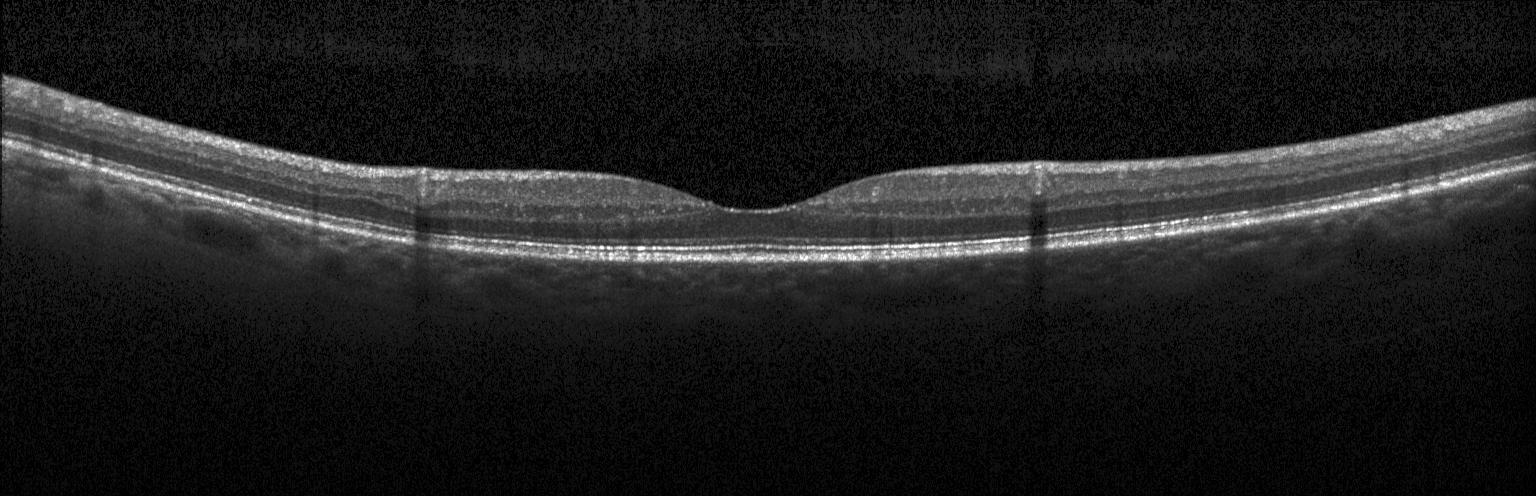 OCT B-scan, horizontal scan through the fovea
Diagnosis: neither choroidal neovascularization, diabetic macular edema, nor drusen.